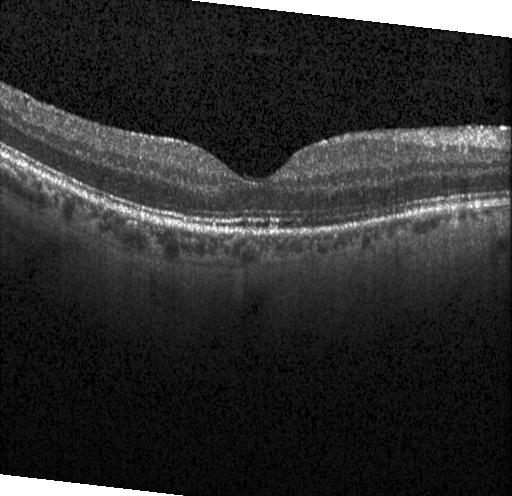

OCT line scan · macular scan · acquired on a Heidelberg Spectralis · SD-OCT
Assessment: neither CNV, DME, nor drusen.